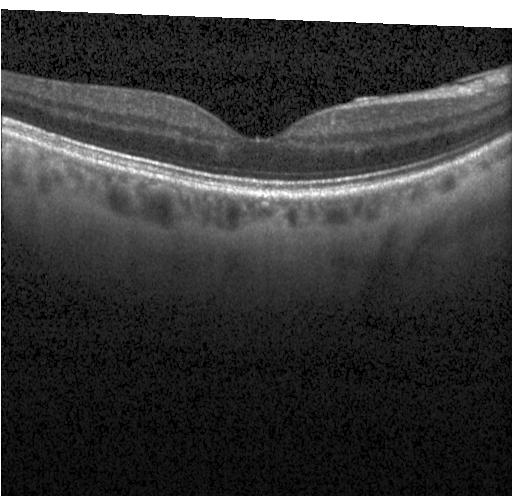 Assessment: no CNV, DME, or drusen.